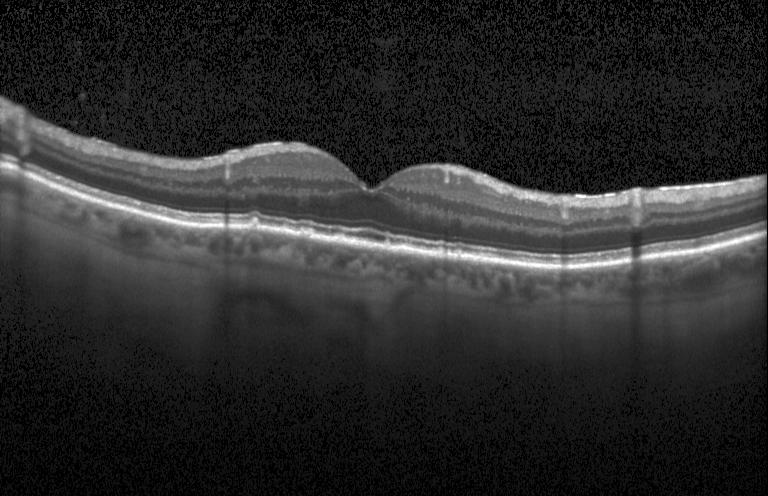 Optical coherence tomography scan.
Diagnosis: sub-RPE drusenoid deposits.